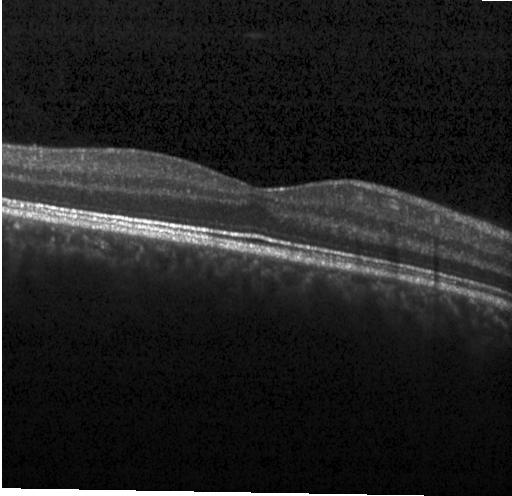 Centered on the fovea. OCT B-scan.
Dx: no choroidal neovascularization, no diabetic macular edema, and no drusen.